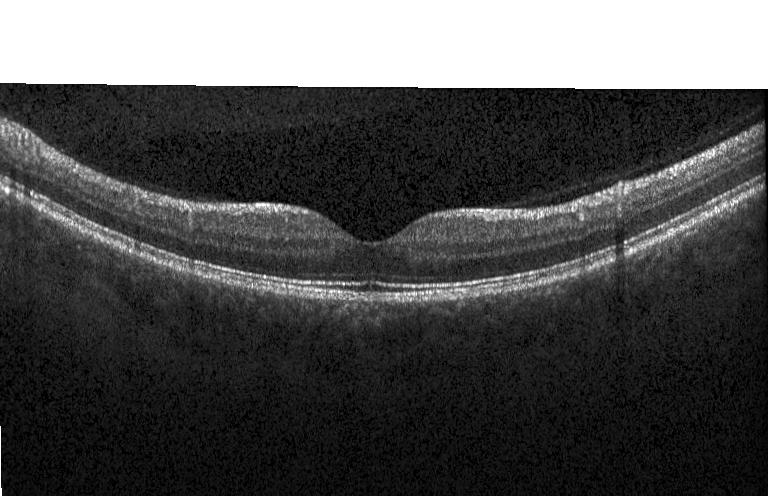 Assessment: no CNV, no DME, and no drusen.